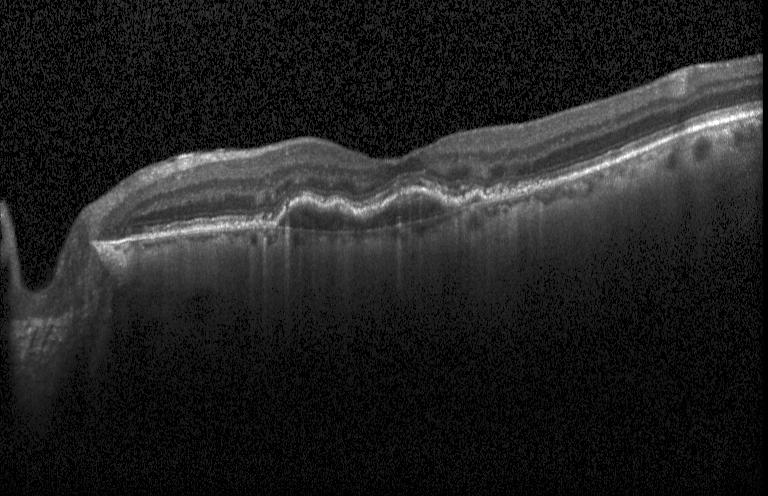
Optical coherence tomography B-scan · macular scan
The scan shows CNV.